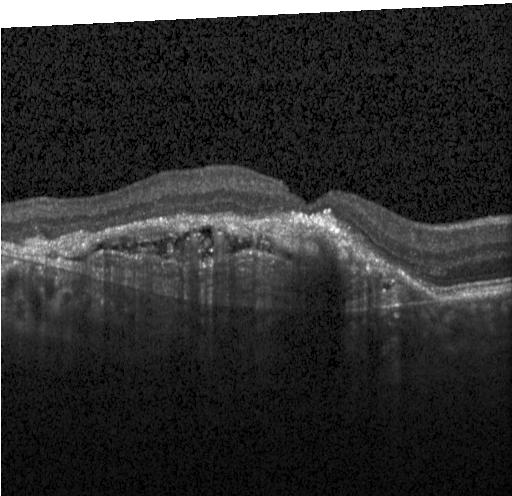
OCT finding: choroidal neovascularization.